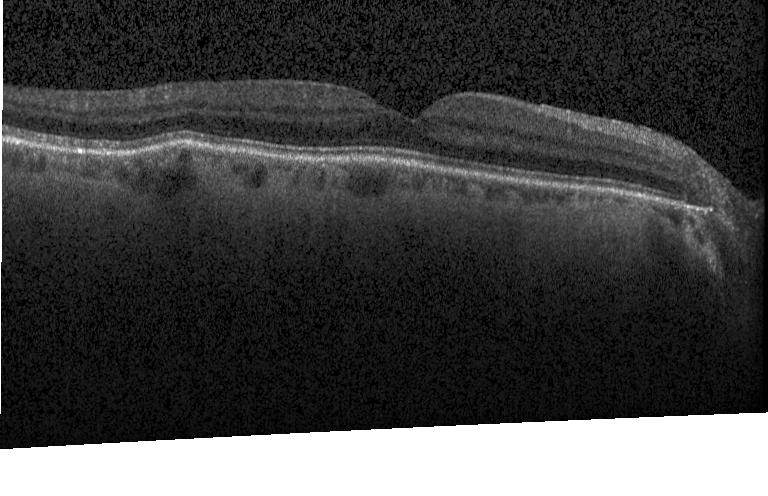 Instrument: Heidelberg Spectralis. OCT B-scan. Spectral-domain OCT. Centered on the fovea. The scan shows no choroidal neovascularization, diabetic macular edema, or drusen.